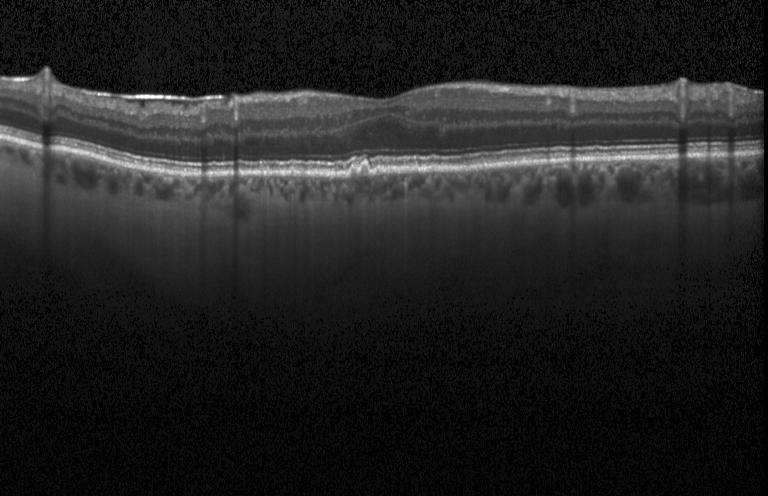

Instrument: Heidelberg Spectralis, SD-OCT, fovea-centered, OCT line scan — Finding: sub-RPE drusenoid deposits.